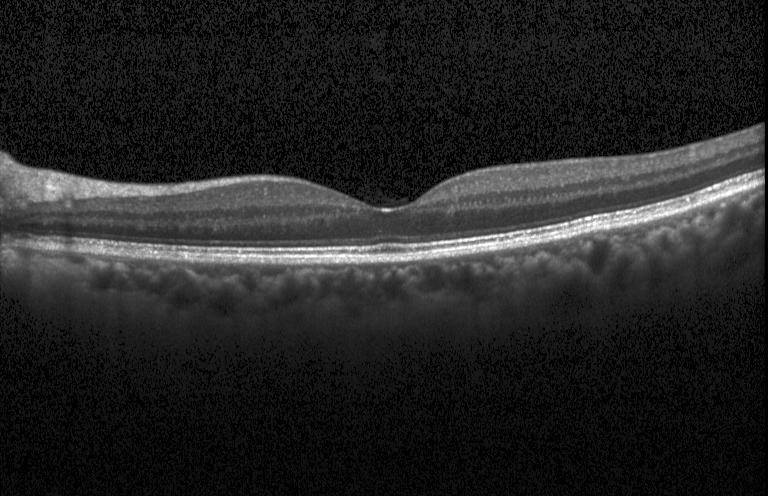 Heidelberg Spectralis OCT system. Fovea-centered. Spectral-domain optical coherence tomography. Retinal OCT cross-section
Impression: neither CNV, DME, nor drusen.